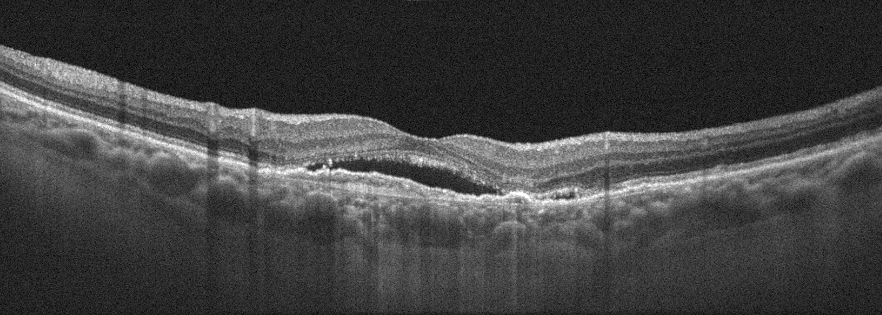
OCT line scan, macular scan, oculus sinister, instrument: Optovue Avanti RTVue XR.
The scan shows age-related macular degeneration (AMD).